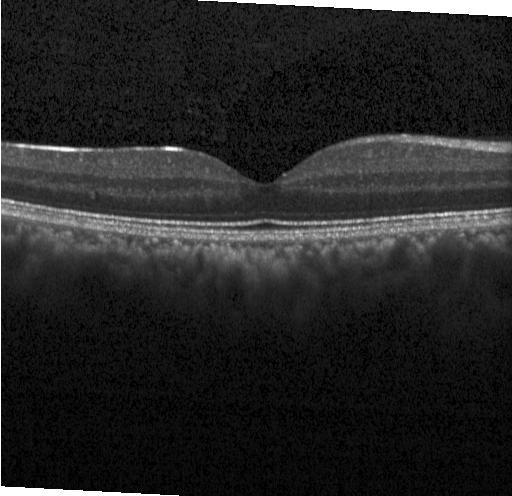
Retinal OCT cross-section showing neither CNV, DME, nor drusen.